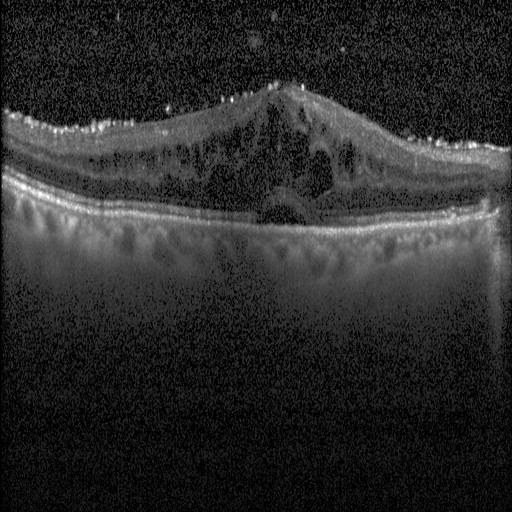

Diagnosis: diabetic macular edema.